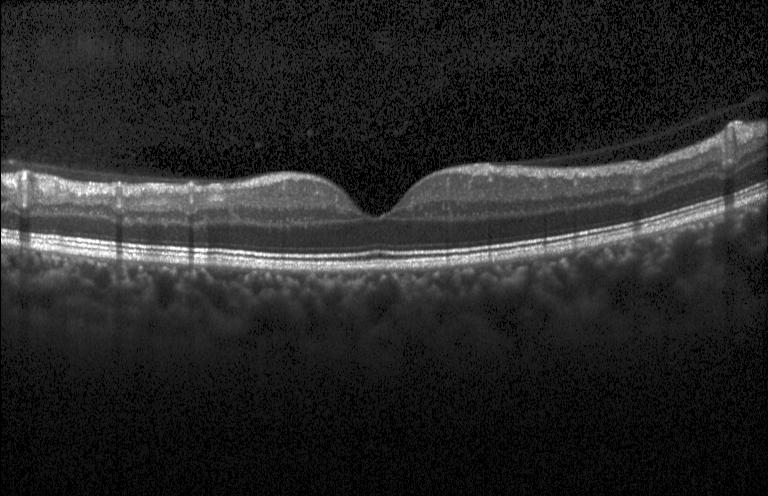

Macular OCT: neither CNV, DME, nor drusen.